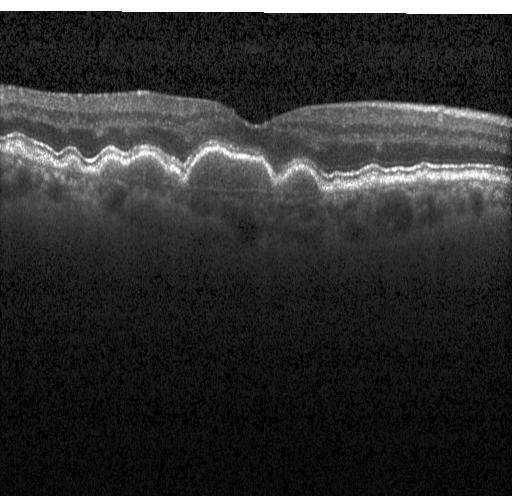 Instrument: Heidelberg Spectralis; optical coherence tomography B-scan; spectral-domain OCT — Sub-RPE drusenoid deposits.